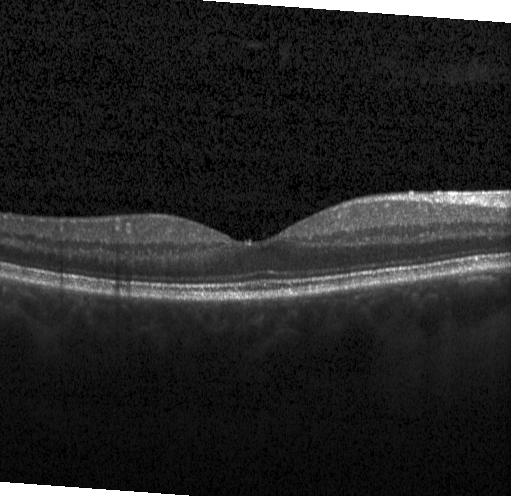
OCT line scan
Impression: neither choroidal neovascularization, diabetic macular edema, nor drusen.